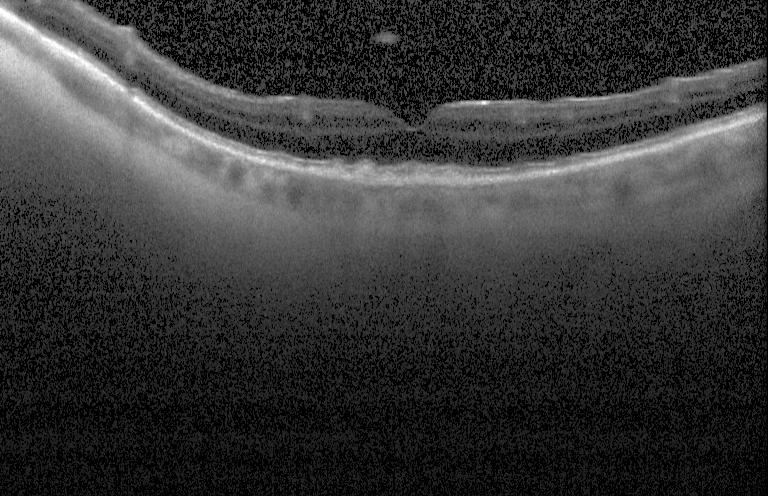 Retinal OCT cross-section — Macular OCT: drusen.